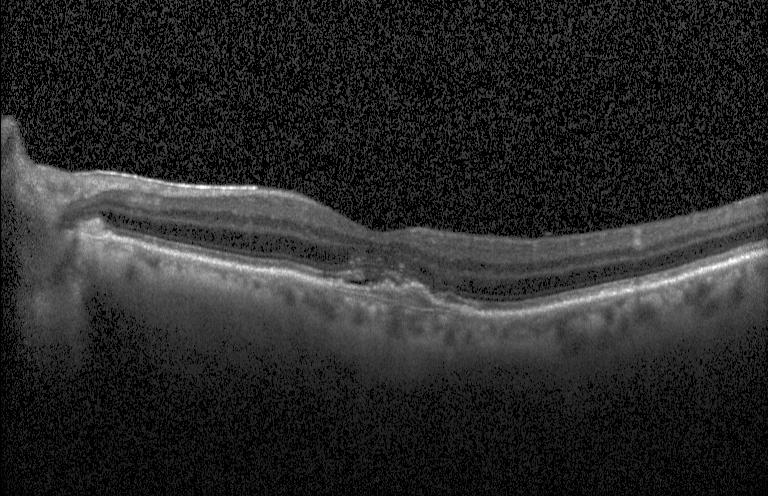
CNV.